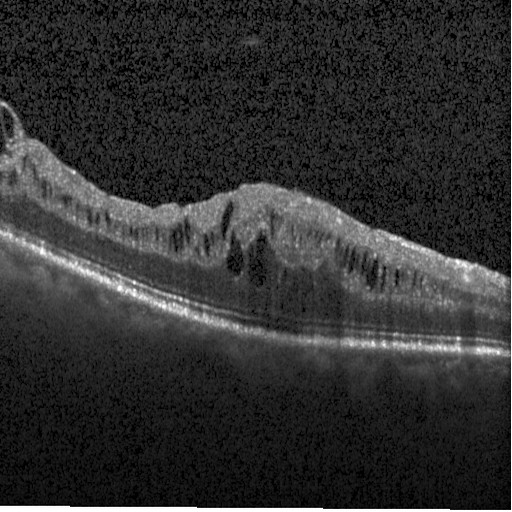
Retinal OCT cross-section.
DME.